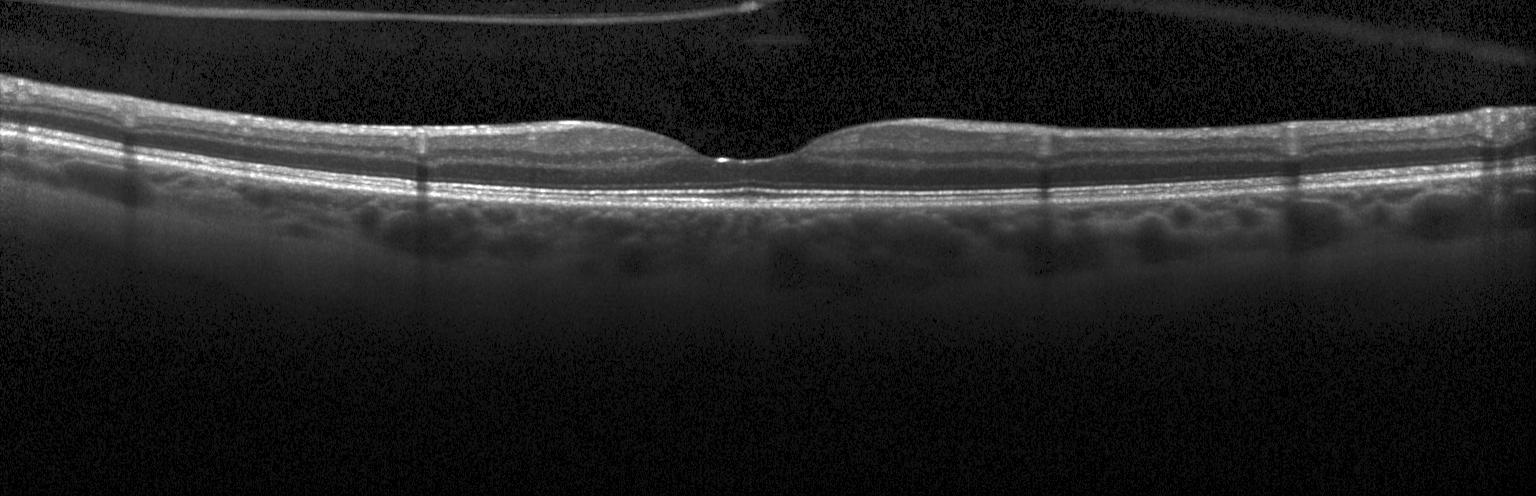 Finding: no CNV, no DME, and no drusen.